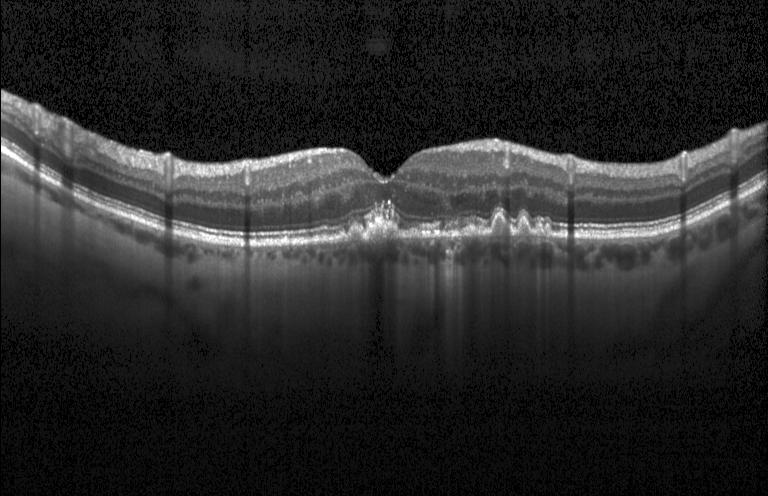
Through the macula; SD-OCT; Heidelberg Spectralis OCT system; optical coherence tomography B-scan. Finding: sub-RPE drusenoid deposits.